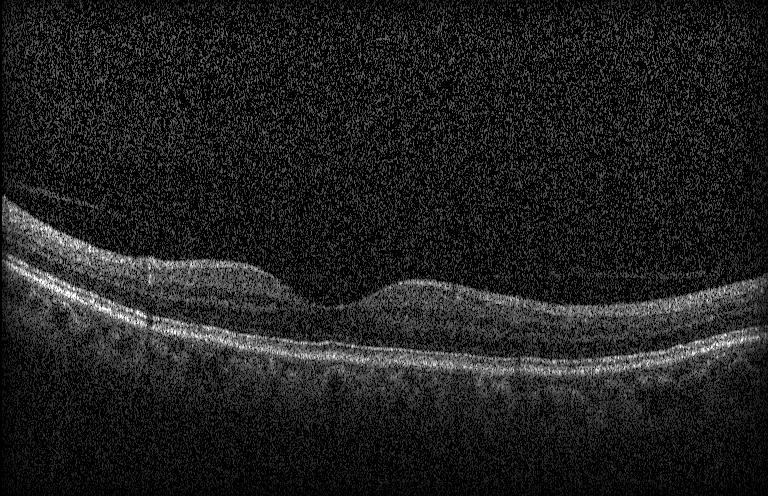
This B-scan demonstrates no evidence of CNV, DME, or drusen.